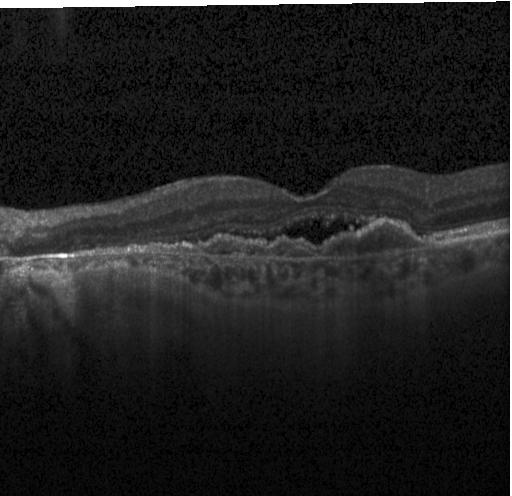
Choroidal neovascularization.